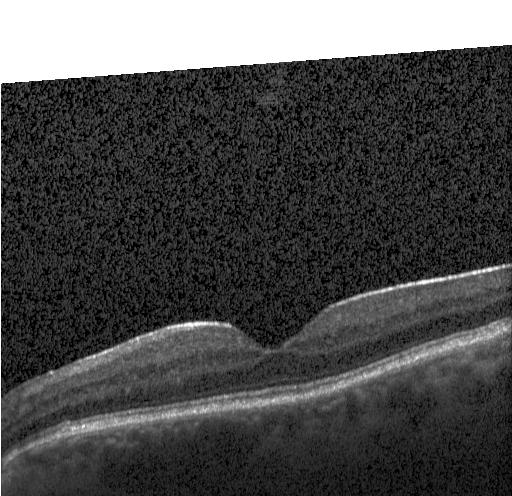
Optical coherence tomography B-scan.
Assessment: no evidence of CNV, DME, or drusen.